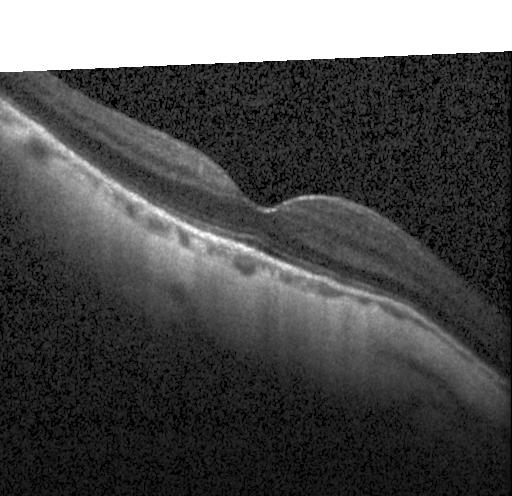
Horizontal scan through the fovea; retinal OCT B-scan; Heidelberg Spectralis OCT system; spectral-domain optical coherence tomography
Diagnosis: no choroidal neovascularization, no diabetic macular edema, and no drusen.